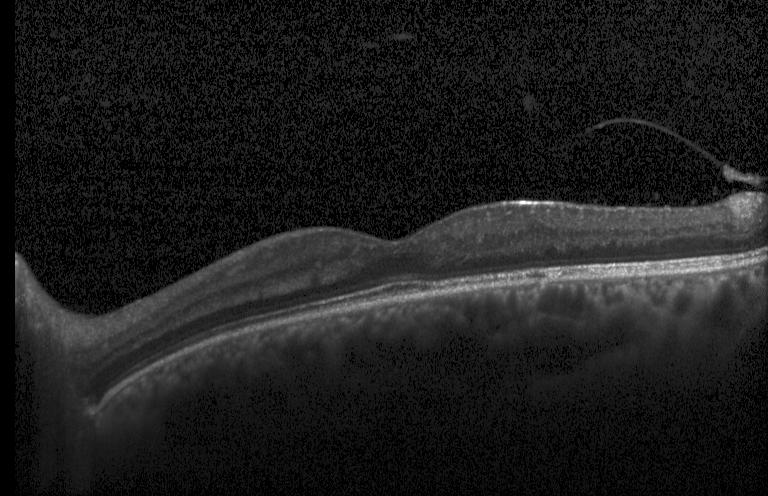
Impression: no CNV, no DME, and no drusen.